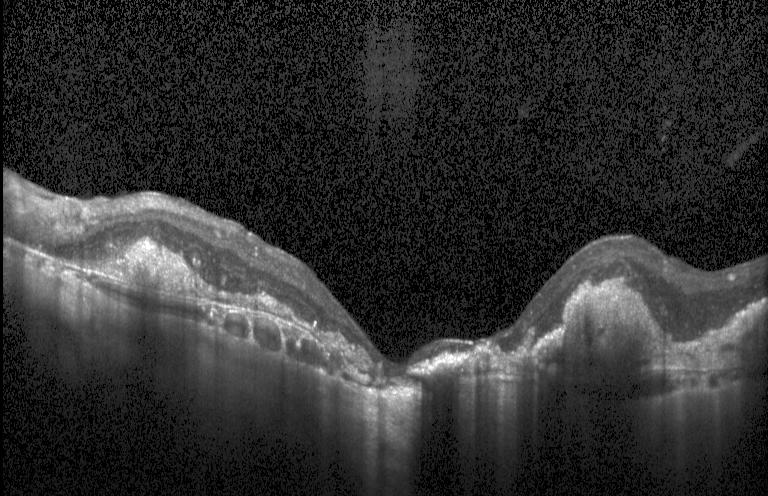

Retinal OCT cross-section — A choroidal neovascular membrane.